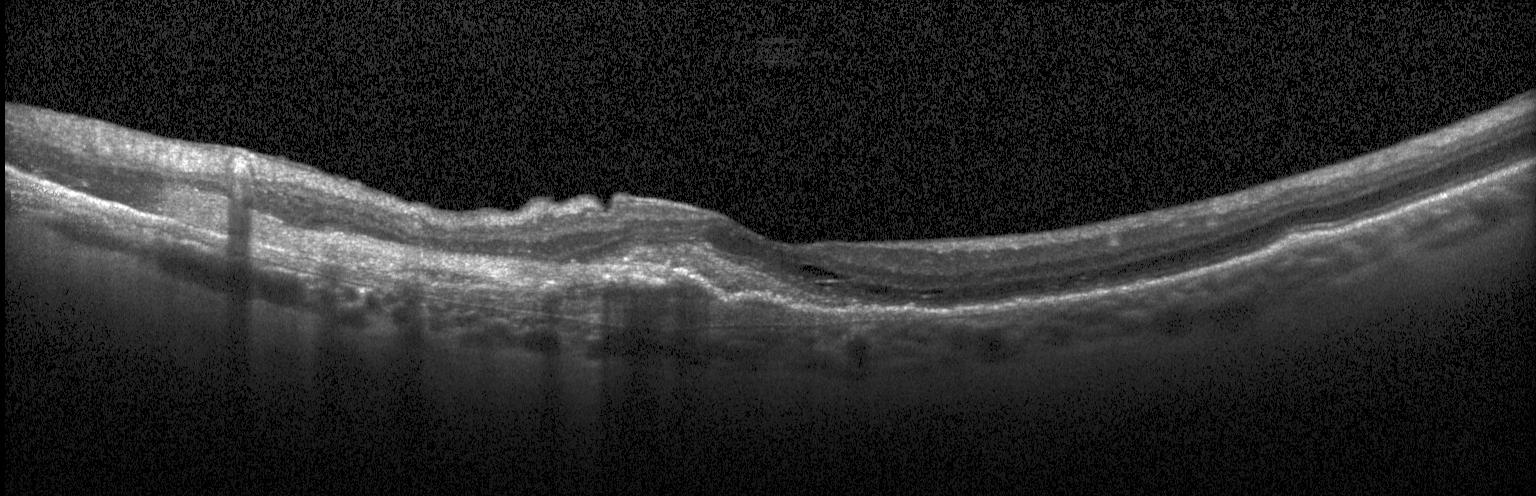
Heidelberg Spectralis OCT system · optical coherence tomography scan. Impression: a choroidal neovascular membrane.